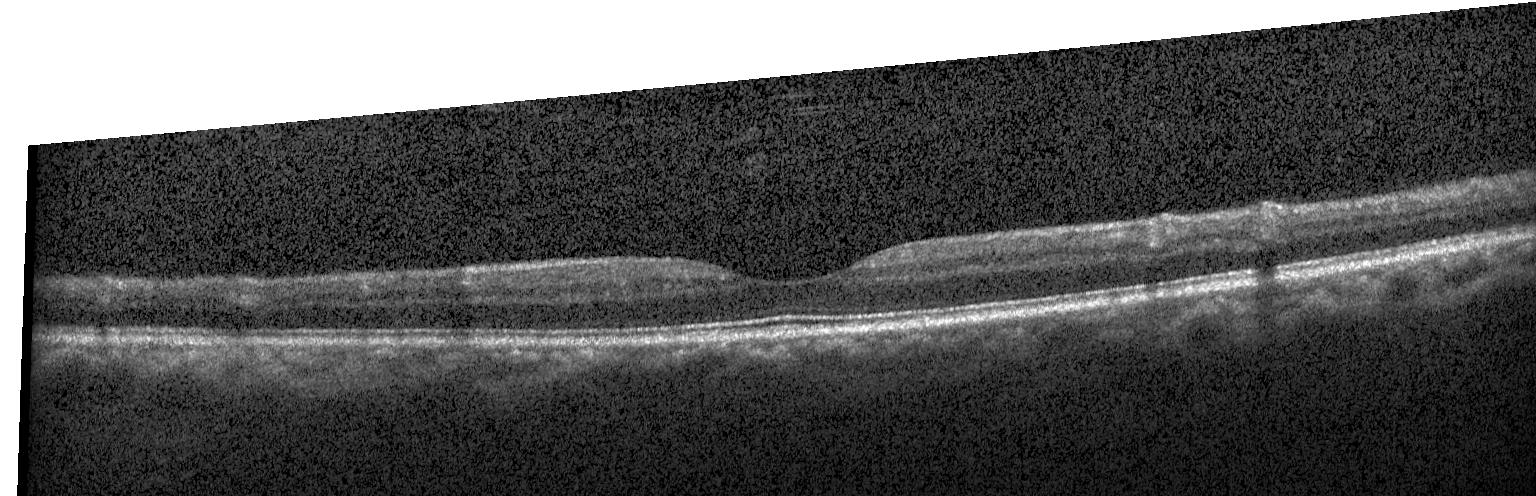

Through the macula. Optical coherence tomography B-scan
Diagnosis: no choroidal neovascularization, diabetic macular edema, or drusen.